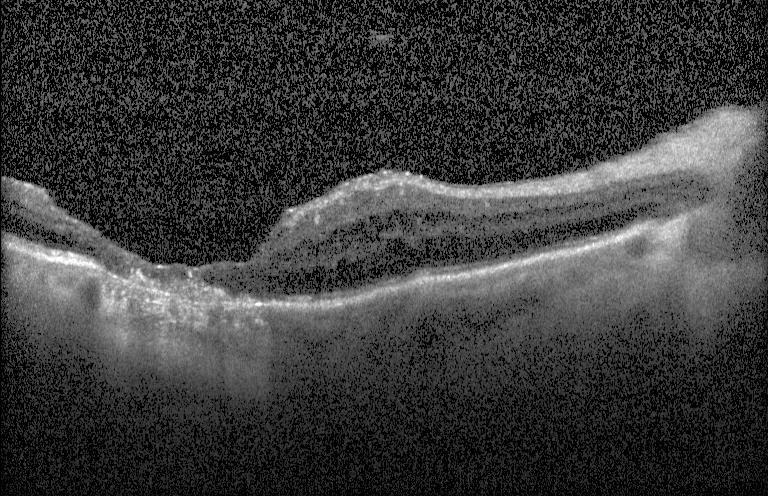
Optical coherence tomography B-scan. Fovea-centered. Spectral-domain optical coherence tomography. Heidelberg Spectralis — Dx: choroidal neovascularization (CNV).